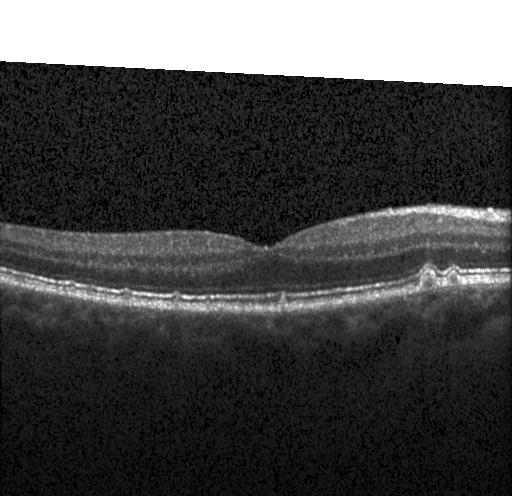
Retinal OCT B-scan — OCT finding: multiple drusen.